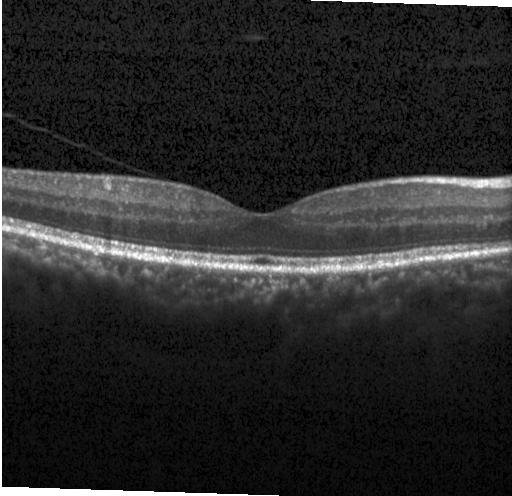 Finding: no CNV, no DME, and no drusen.